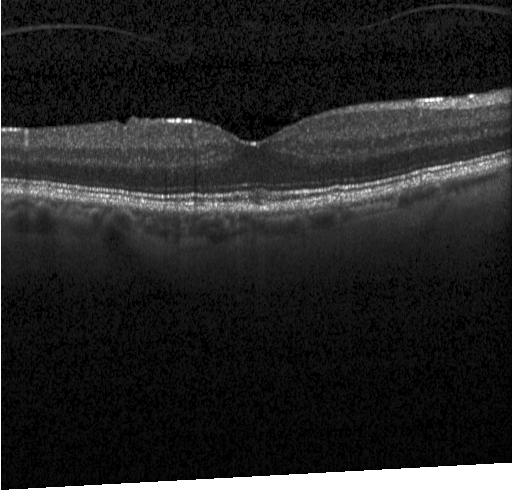
Instrument: Heidelberg Spectralis; fovea-centered; spectral-domain optical coherence tomography; optical coherence tomography B-scan — Finding: no choroidal neovascularization, diabetic macular edema, or drusen.